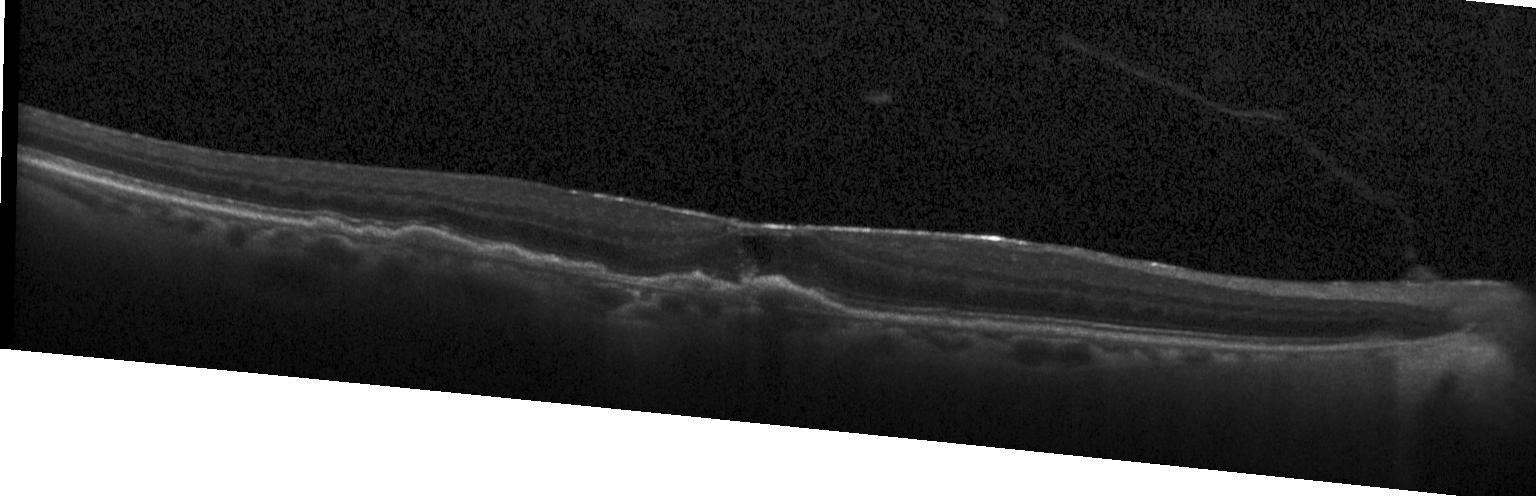
SD-OCT, retinal OCT B-scan — Diagnosis: a choroidal neovascular membrane.